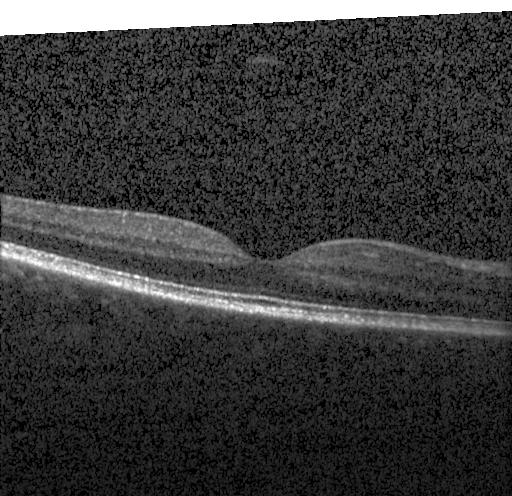
Spectral-domain optical coherence tomography · macular scan · optical coherence tomography scan — Impression: no choroidal neovascularization, diabetic macular edema, or drusen.